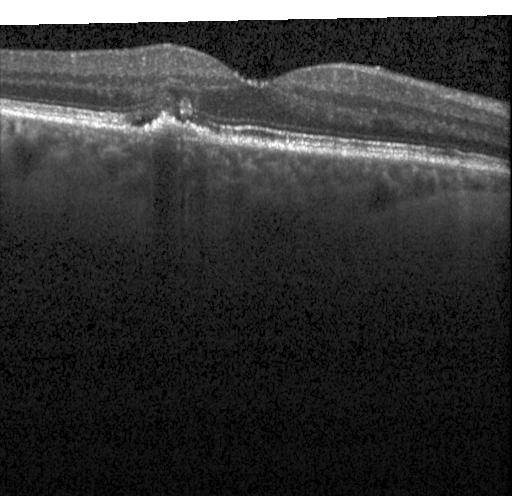 Horizontal scan through the fovea, OCT B-scan, acquired on a Heidelberg Spectralis, spectral-domain OCT — OCT finding: a choroidal neovascular membrane.